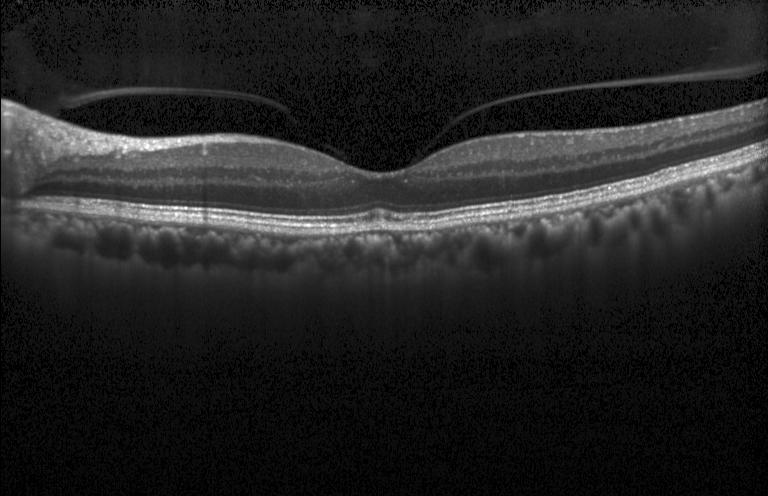 Optical coherence tomography B-scan.
Finding: neither CNV, DME, nor drusen.